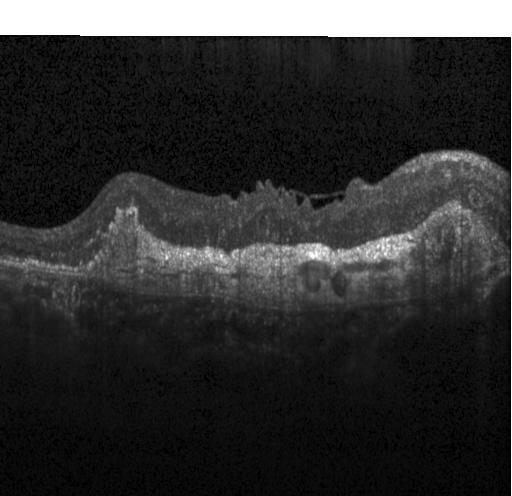
Retinal OCT cross-section, spectral-domain OCT, Heidelberg Spectralis OCT system — This B-scan demonstrates choroidal neovascularization.